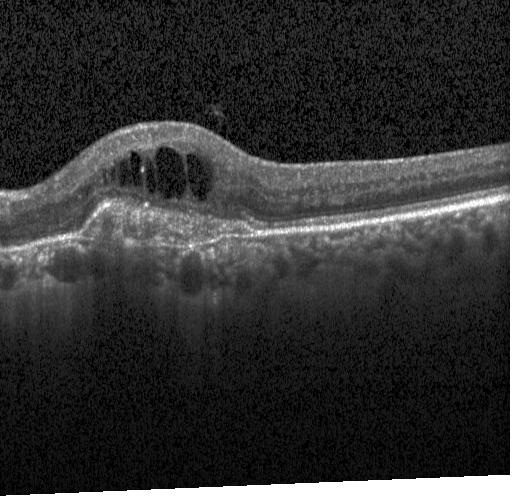

Macular OCT demonstrating a choroidal neovascular membrane.